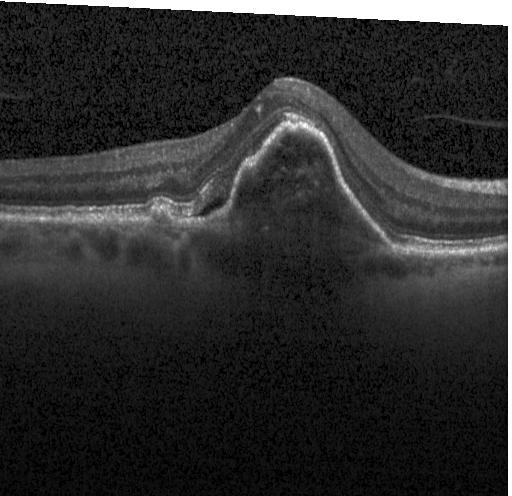

Optical coherence tomography scan
Finding: choroidal neovascularization (CNV).